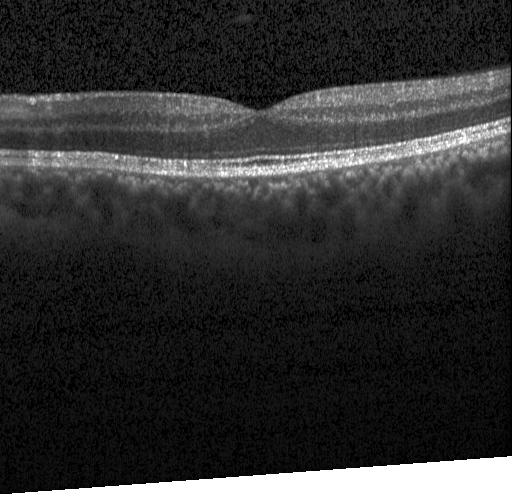
Optical coherence tomography scan
Impression: no CNV, DME, or drusen.